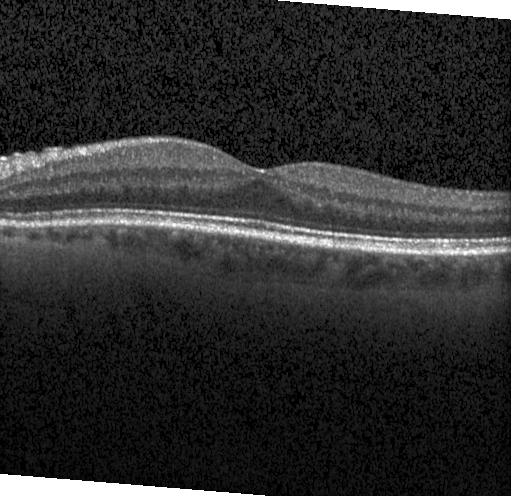
Retinal OCT cross-section
Diagnosis: no choroidal neovascularization, diabetic macular edema, or drusen.